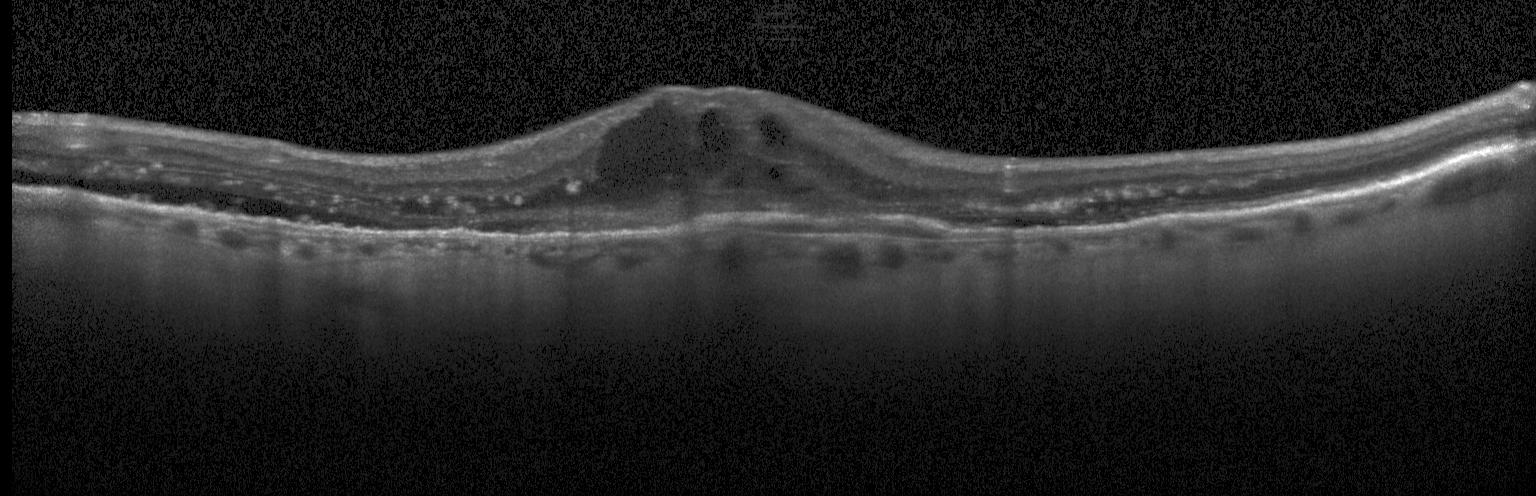

Fovea-centered, spectral-domain OCT, instrument: Heidelberg Spectralis, retinal OCT cross-section — Macular OCT: a choroidal neovascular membrane.